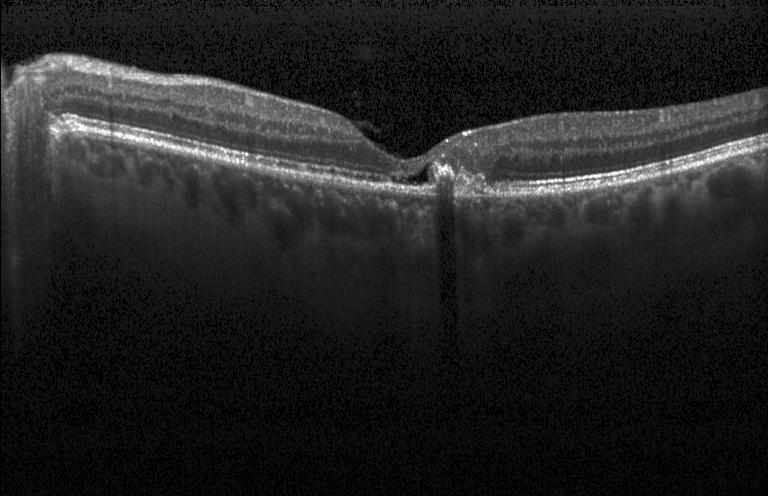 Retinal OCT B-scan. Spectral-domain optical coherence tomography. Finding: choroidal neovascularization.